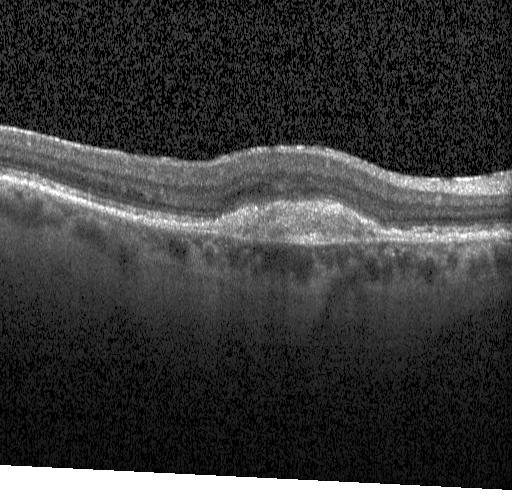

Fovea-centered · optical coherence tomography B-scan. Assessment: choroidal neovascularization.